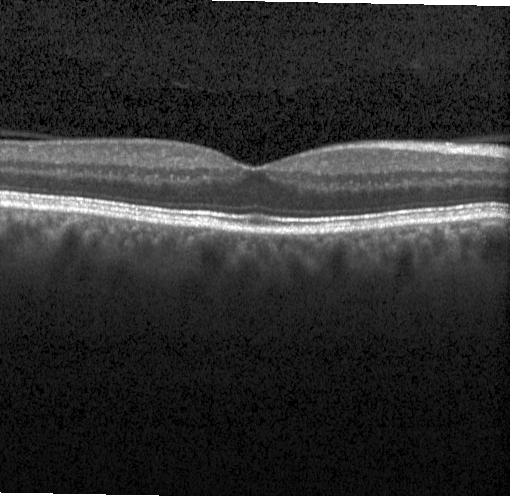
OCT scan showing no choroidal neovascularization, diabetic macular edema, or drusen.